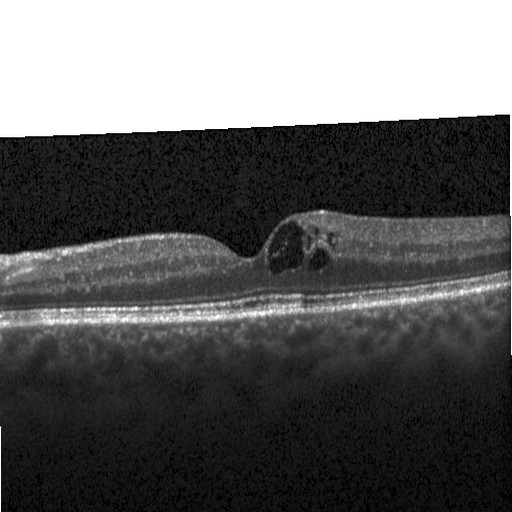 Assessment: DME.